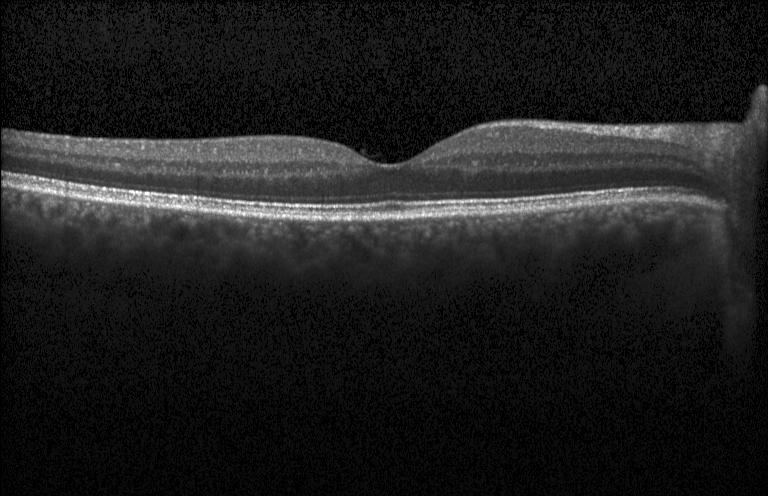 OCT B-scan, spectral-domain optical coherence tomography, instrument: Heidelberg Spectralis.
The scan shows no evidence of CNV, DME, or drusen.